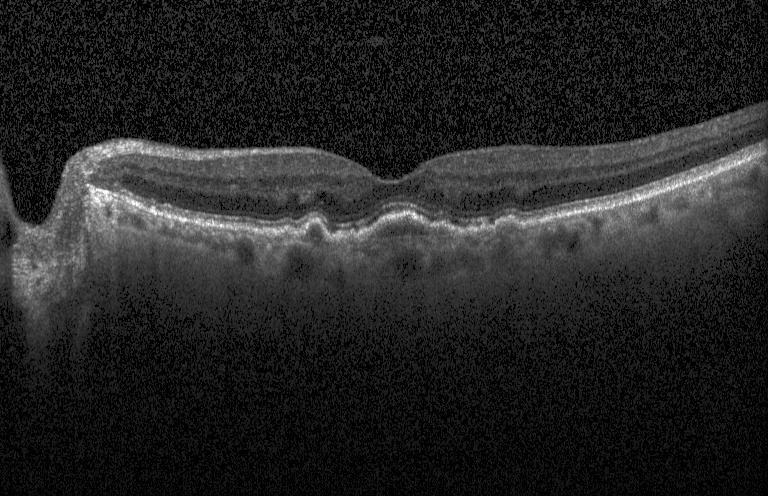

Optical coherence tomography B-scan, spectral-domain optical coherence tomography, Heidelberg Spectralis OCT system, macular scan.
Finding: a choroidal neovascular membrane.